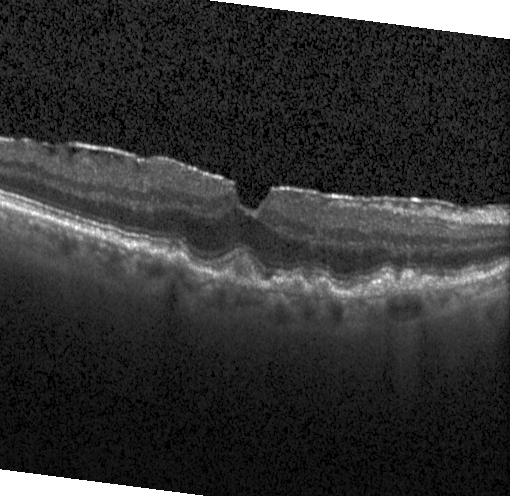
Diagnosis: multiple drusen.